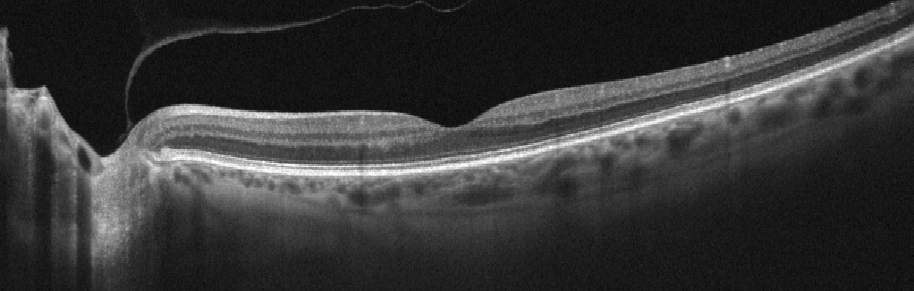
OD; retinal OCT B-scan — OCT finding: absence of AMD, DME, ERM, RAO, RVO, and vitreomacular interface disease.